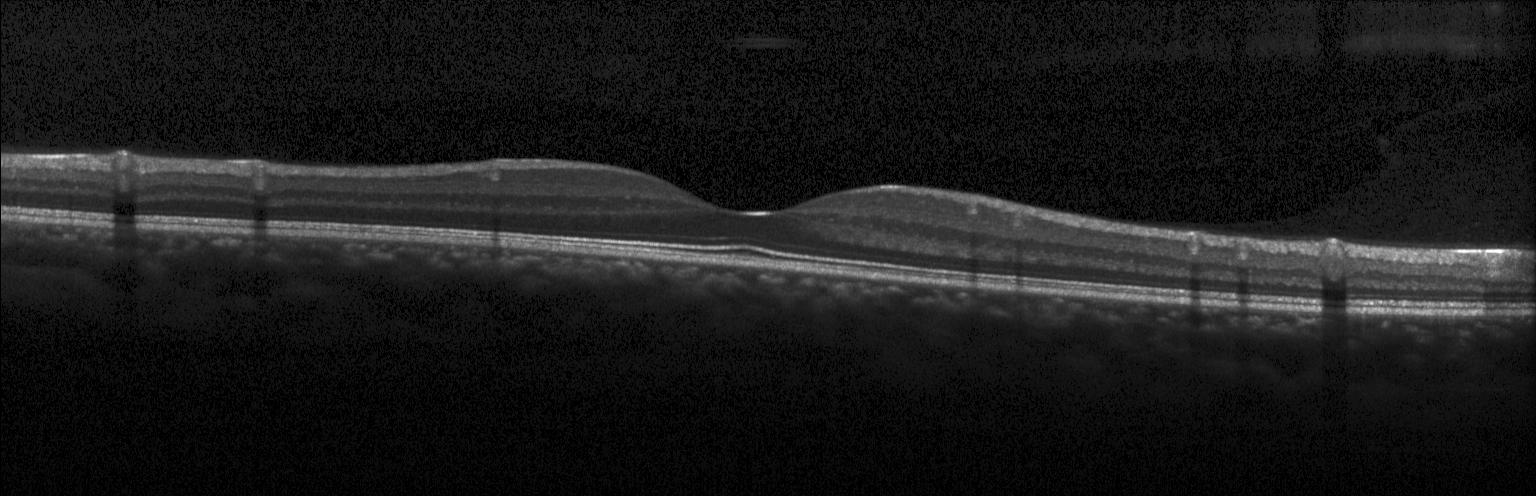

Finding: no evidence of choroidal neovascularization, diabetic macular edema, or drusen.